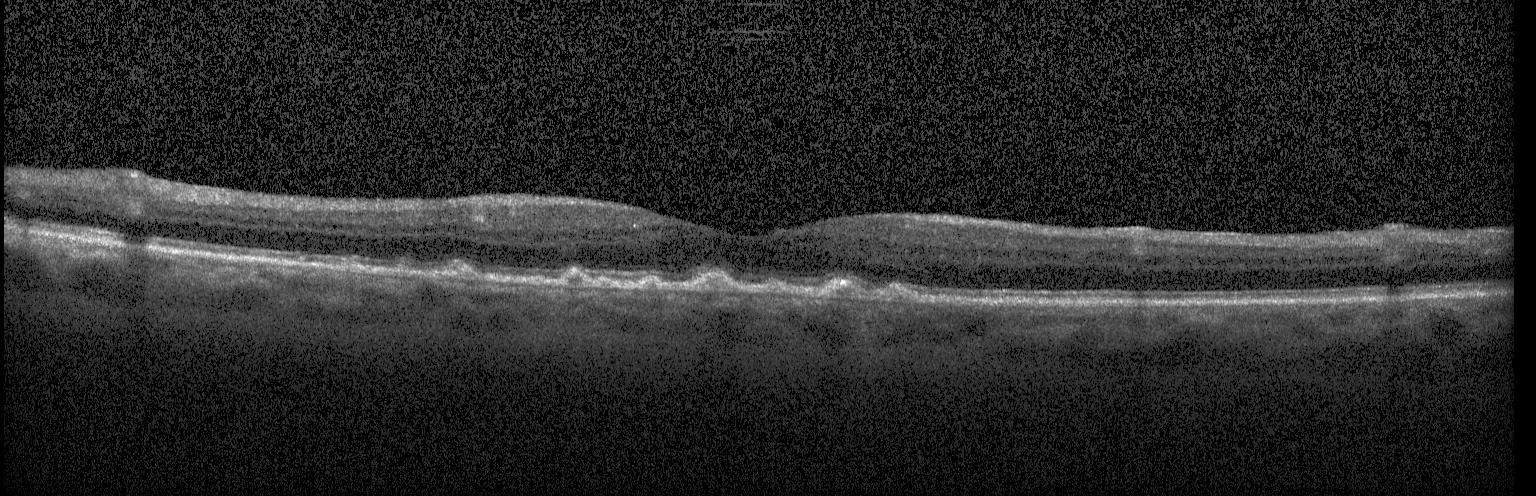

Through the macula, spectral-domain OCT, optical coherence tomography scan.
Sub-RPE drusenoid deposits.